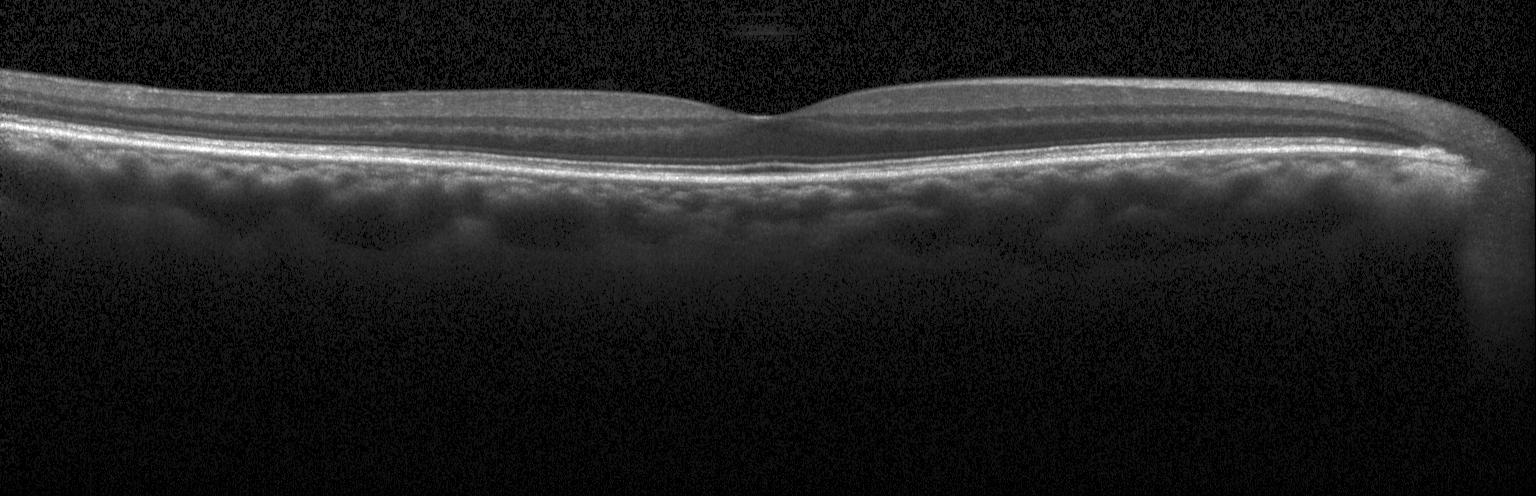

Diagnosis: no evidence of choroidal neovascularization, diabetic macular edema, or drusen.